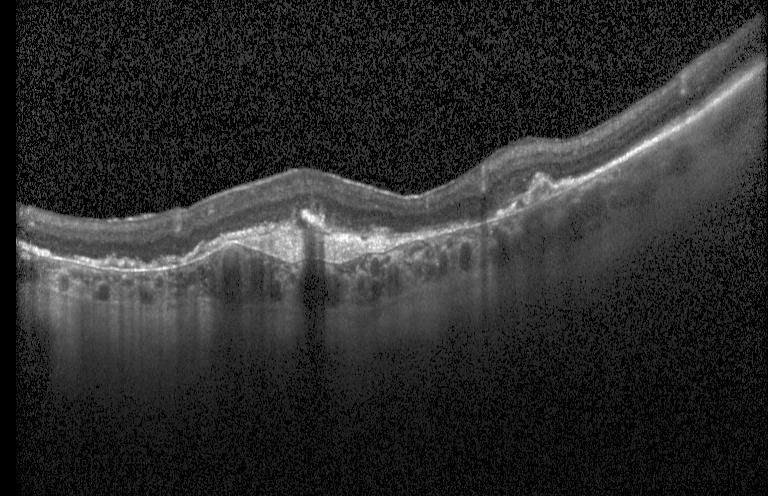

Macular OCT demonstrating choroidal neovascularization (CNV).